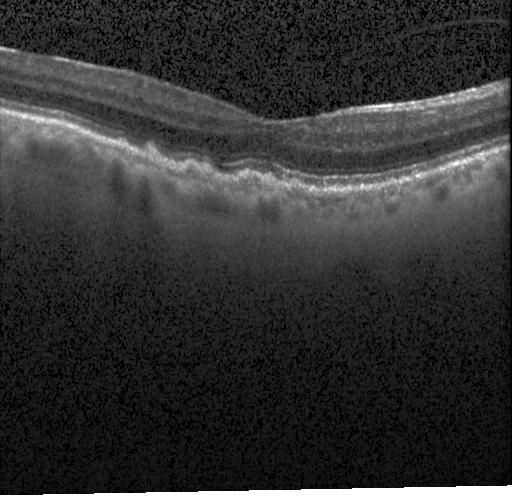

OCT B-scan showing sub-RPE drusenoid deposits.